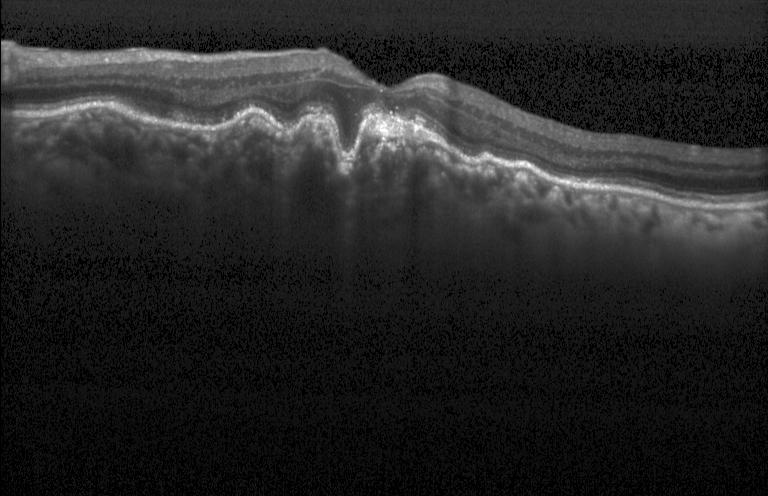
Instrument: Heidelberg Spectralis, OCT line scan
Finding: a choroidal neovascular membrane.